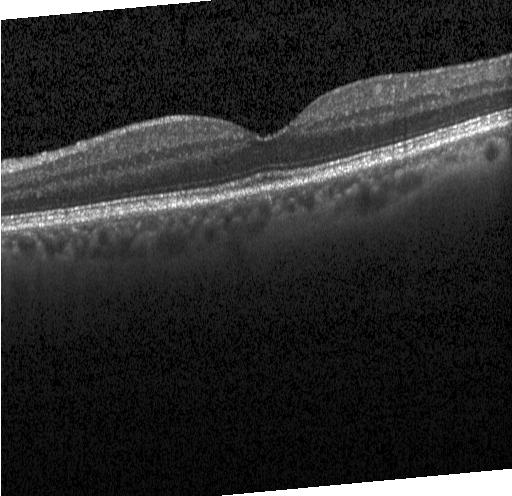 Impression: no evidence of choroidal neovascularization, diabetic macular edema, or drusen.